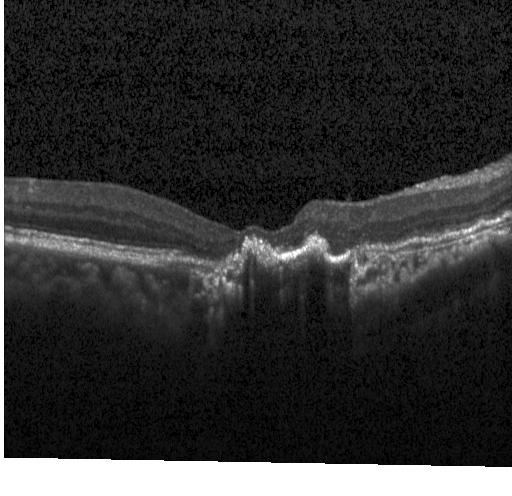

Acquired on a Heidelberg Spectralis. OCT line scan. Spectral-domain OCT
Impression: choroidal neovascularization.